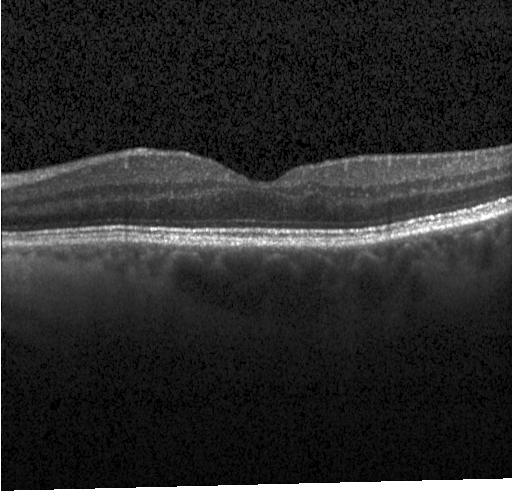
Retinal OCT B-scan, instrument: Heidelberg Spectralis.
Diagnosis: no evidence of CNV, DME, or drusen.